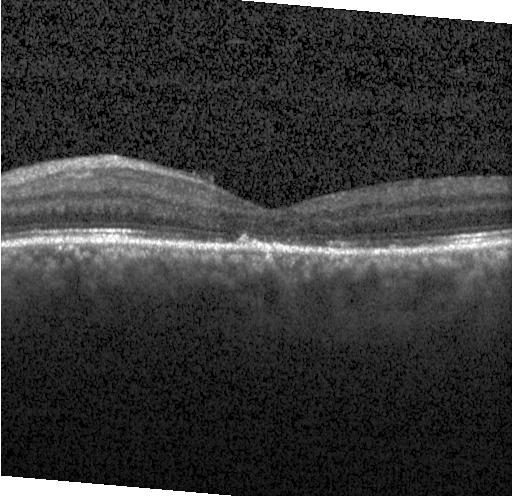 Macular OCT: multiple drusen.